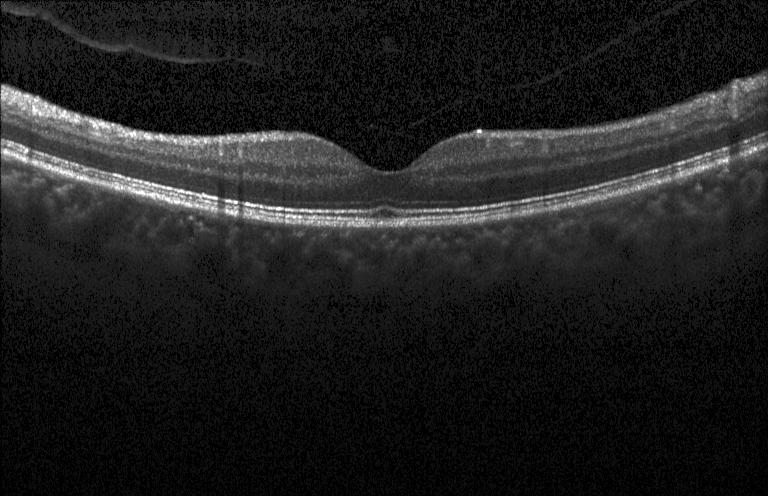 This B-scan demonstrates no choroidal neovascularization, diabetic macular edema, or drusen.